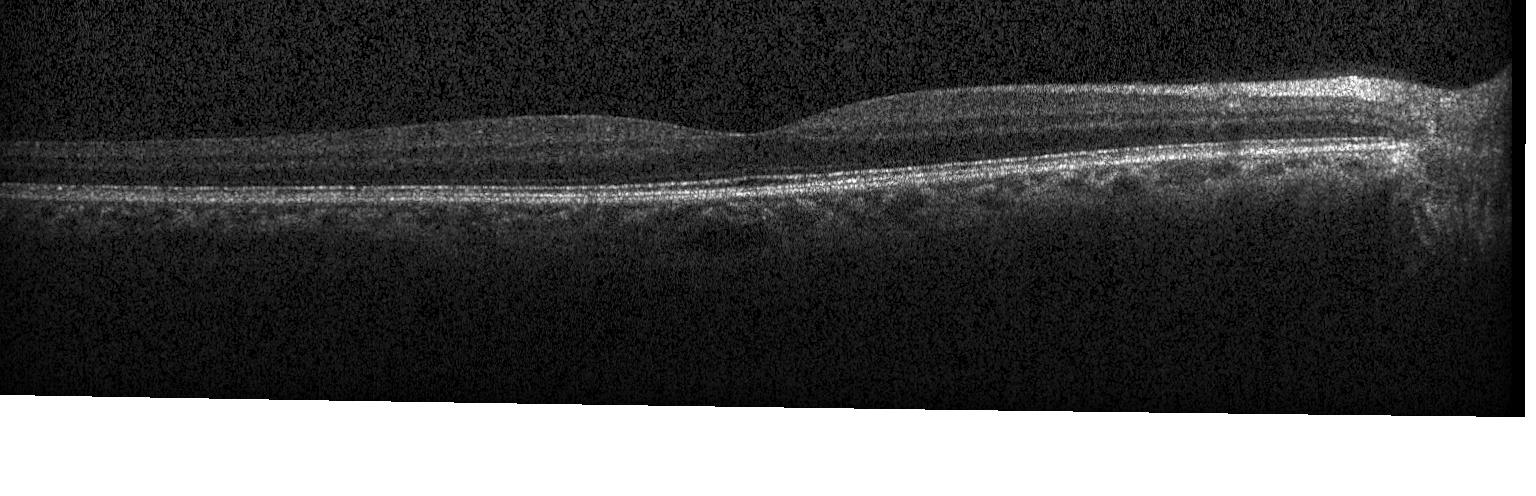 Assessment: no CNV, DME, or drusen.